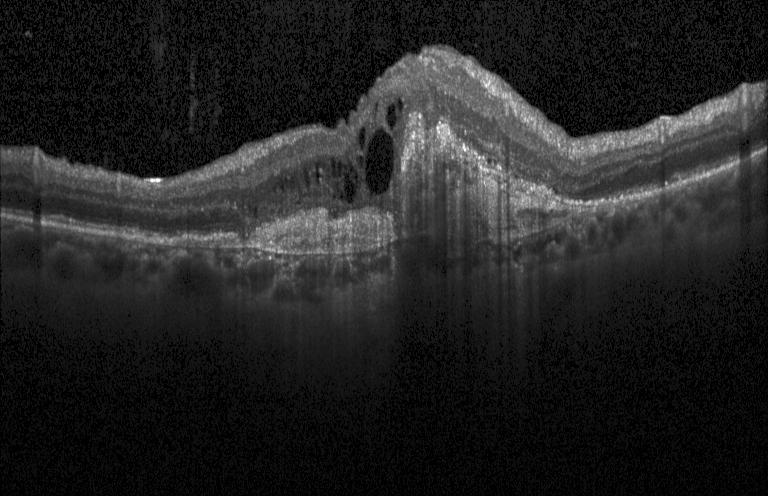
Optical coherence tomography B-scan
Diagnosis: choroidal neovascularization (CNV).